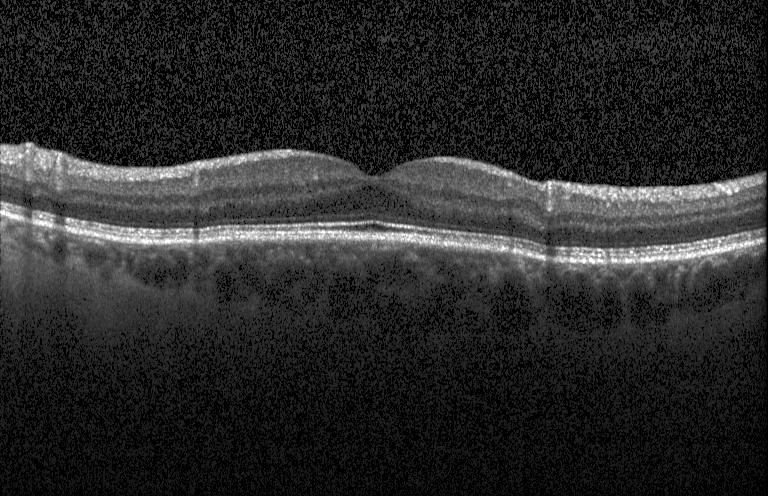

OCT B-scan — No choroidal neovascularization, diabetic macular edema, or drusen.